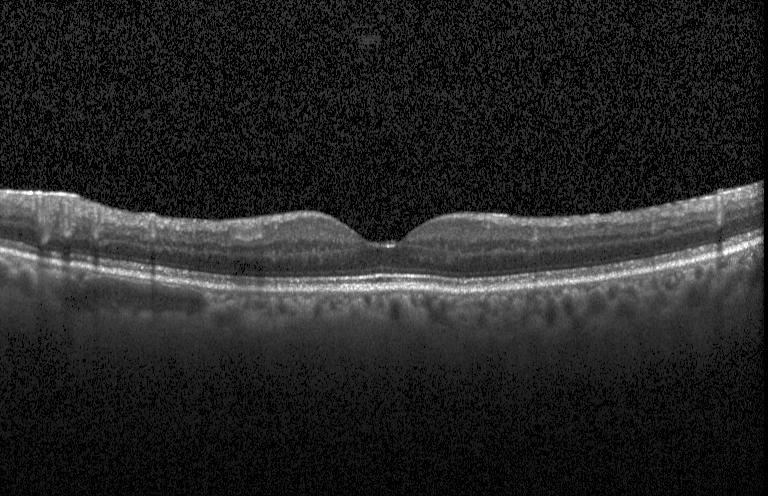

Retinal OCT B-scan — Assessment: no choroidal neovascularization, diabetic macular edema, or drusen.